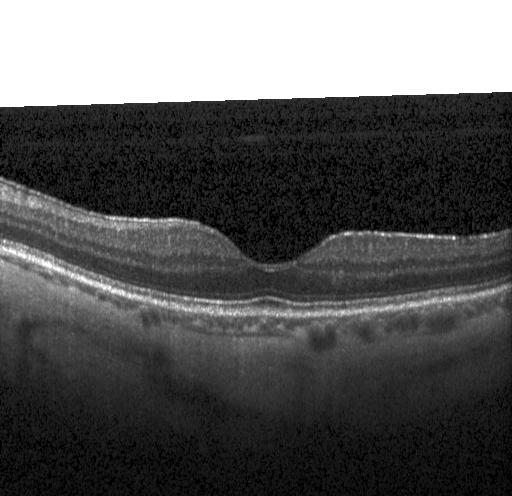 Spectral-domain optical coherence tomography, acquired on a Heidelberg Spectralis, optical coherence tomography B-scan
Macular OCT: no choroidal neovascularization, diabetic macular edema, or drusen.